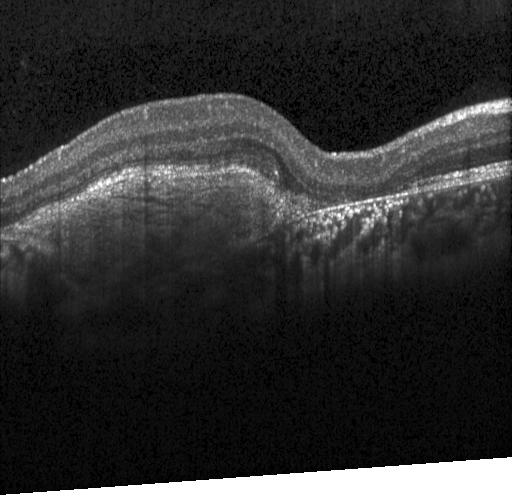 Diagnosis: choroidal neovascularization.